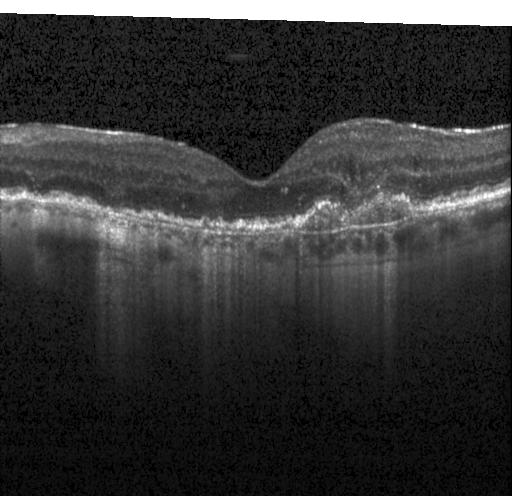

Optical coherence tomography B-scan. The scan shows CNV.